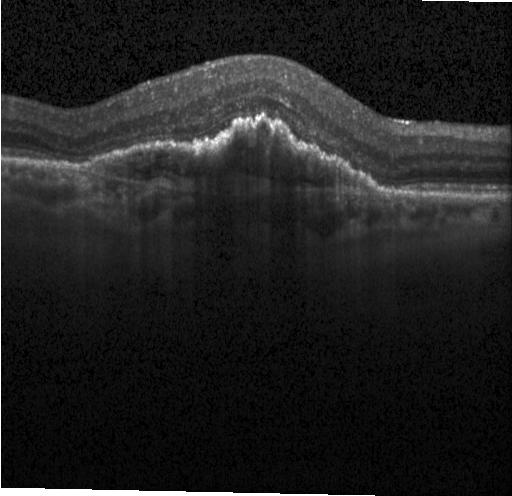 OCT B-scan showing a choroidal neovascular membrane.